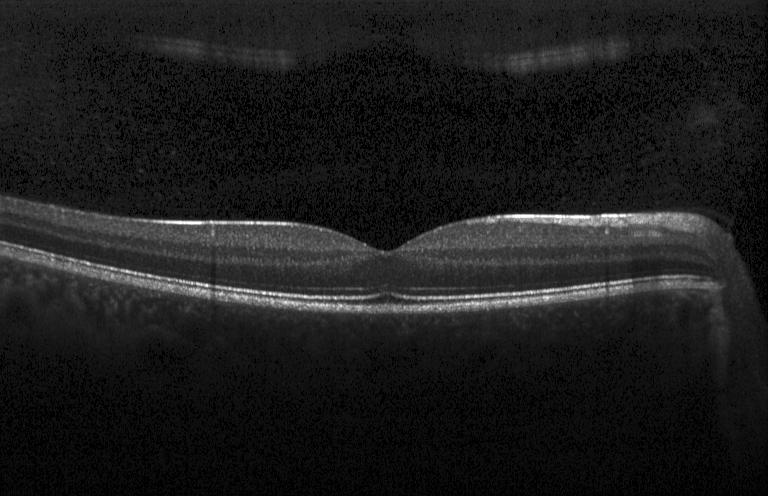 Spectral-domain optical coherence tomography; OCT line scan; Heidelberg Spectralis OCT system.
Macular OCT: no evidence of CNV, DME, or drusen.